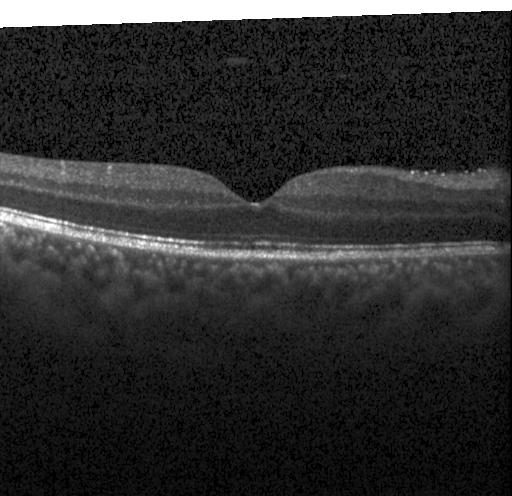

Diagnosis: no evidence of choroidal neovascularization, diabetic macular edema, or drusen.